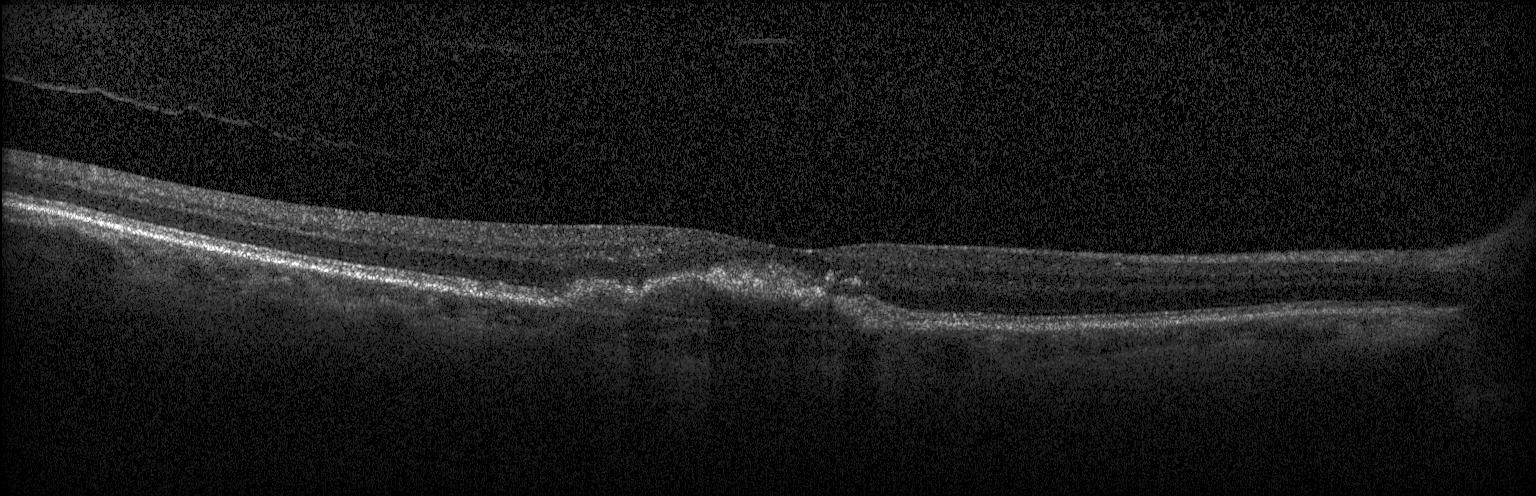 Macular OCT demonstrating choroidal neovascularization.